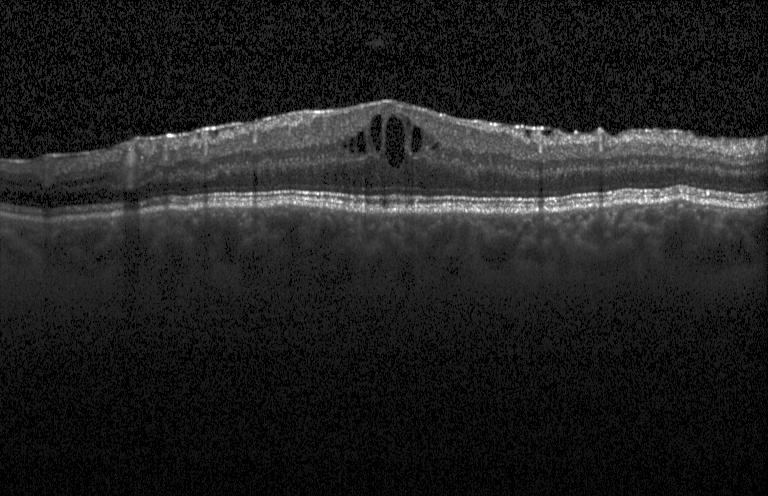 Retinal OCT cross-section.
Dx: DME.